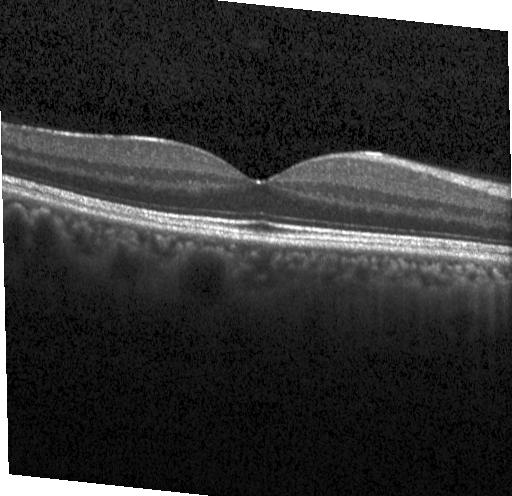

OCT finding: neither choroidal neovascularization, diabetic macular edema, nor drusen.